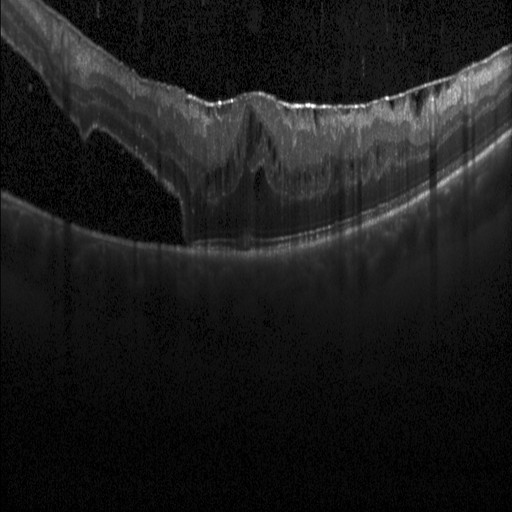
Retinal OCT cross-section — This B-scan demonstrates diabetic macular edema (DME).